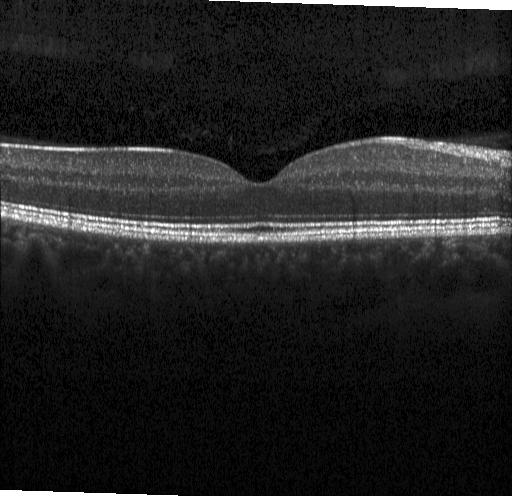 OCT B-scan showing no CNV, DME, or drusen.